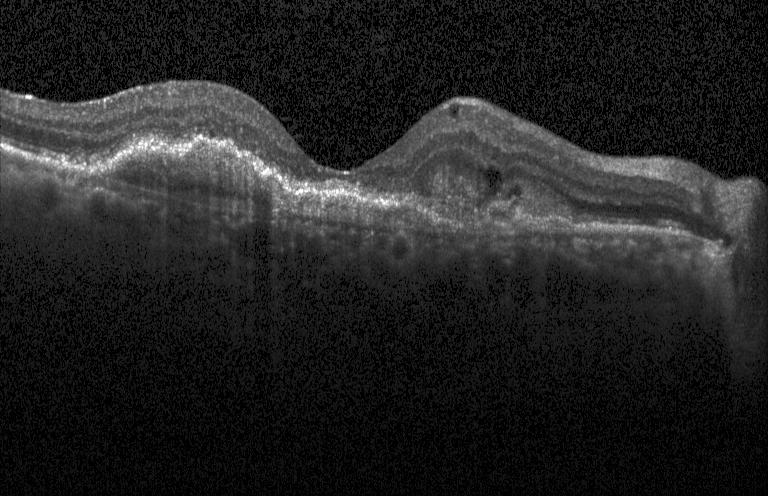

Centered on the fovea; optical coherence tomography B-scan.
This B-scan demonstrates a choroidal neovascular membrane.